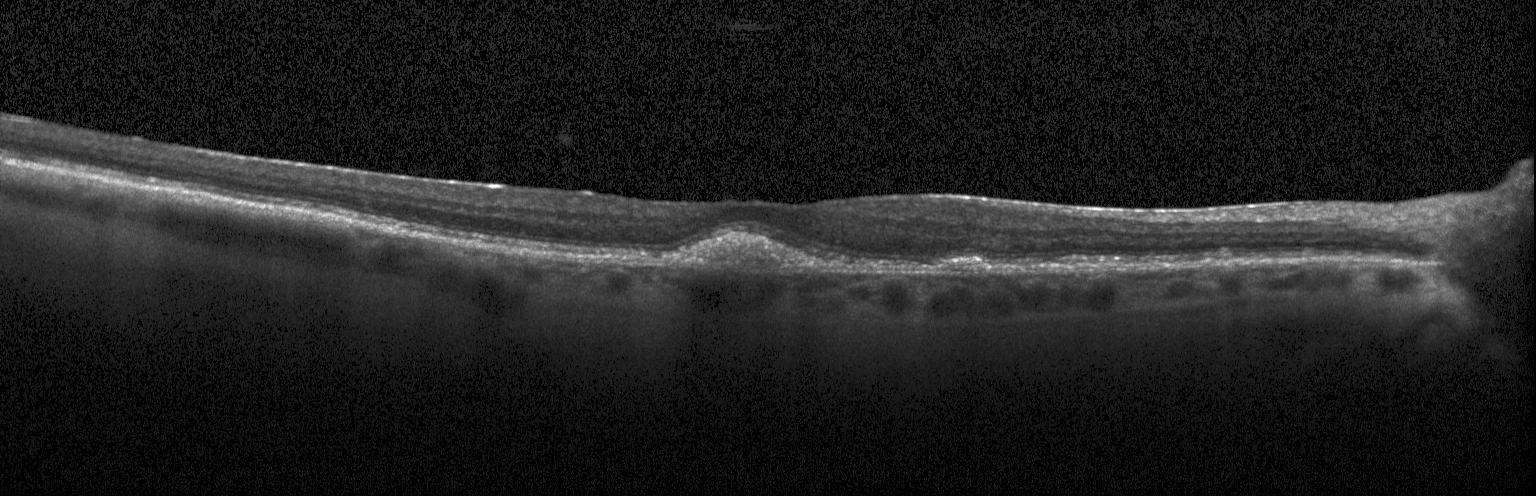
Fovea-centered; SD-OCT; retinal OCT cross-section
Finding: choroidal neovascularization.